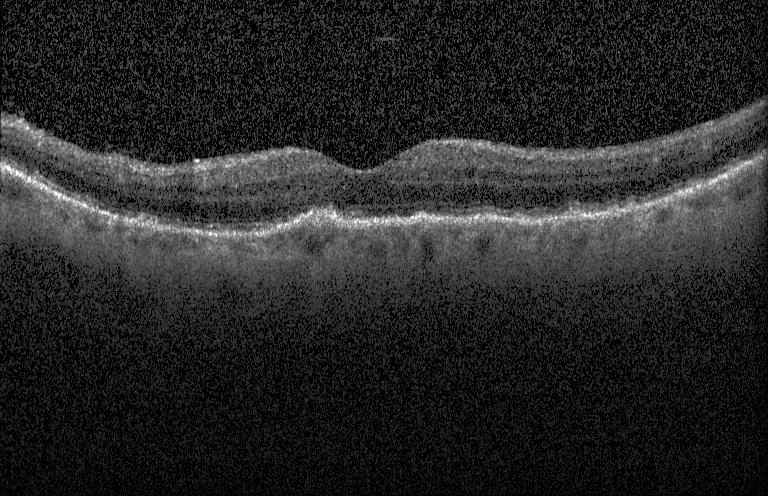

Retinal OCT B-scan. Fovea-centered.
Impression: a choroidal neovascular membrane.